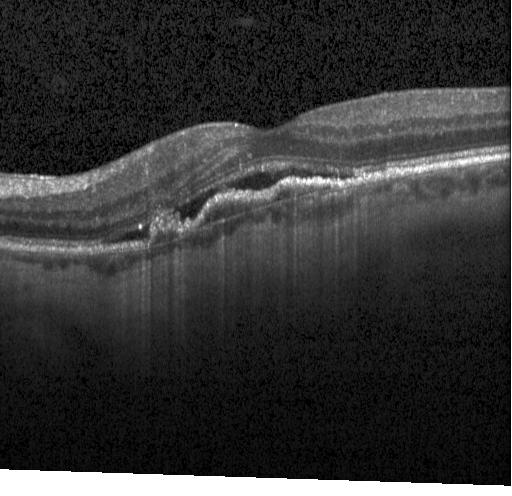
Impression: a choroidal neovascular membrane.